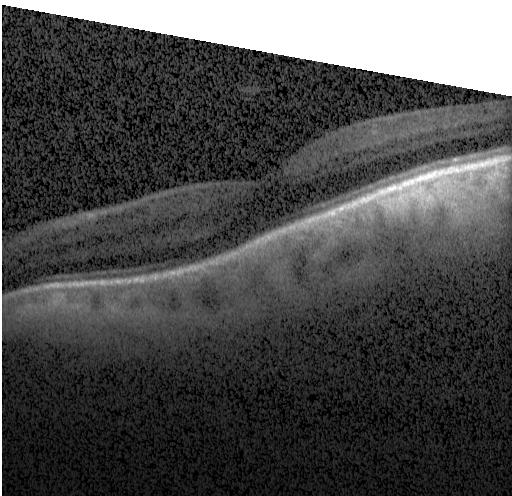

OCT scan showing no choroidal neovascularization, diabetic macular edema, or drusen.